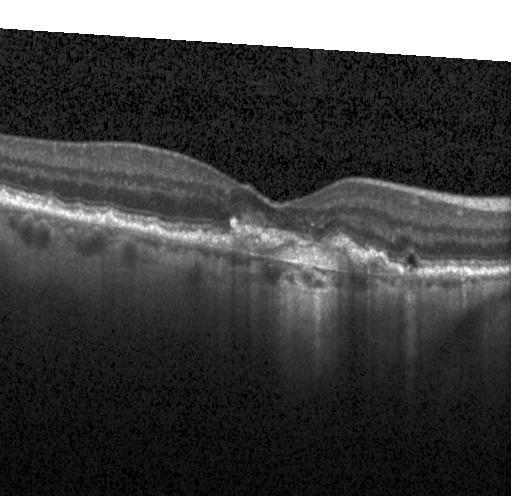

Retinal OCT B-scan.
Impression: choroidal neovascularization.